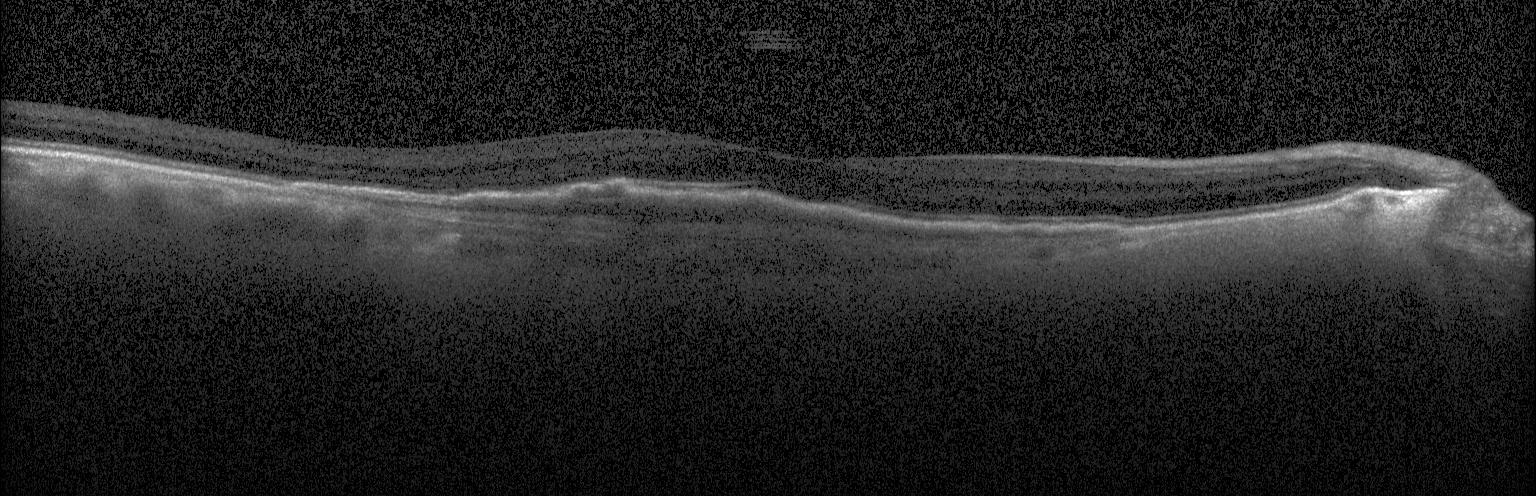 Impression: a choroidal neovascular membrane.